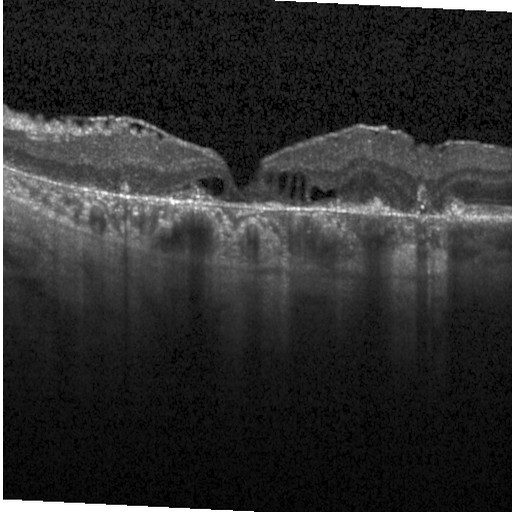
Macular OCT demonstrating DME.